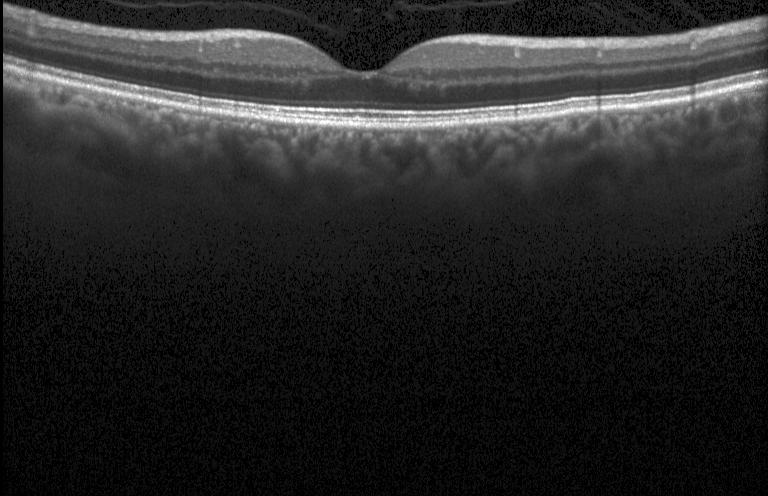

Macular OCT demonstrating no CNV, no DME, and no drusen.